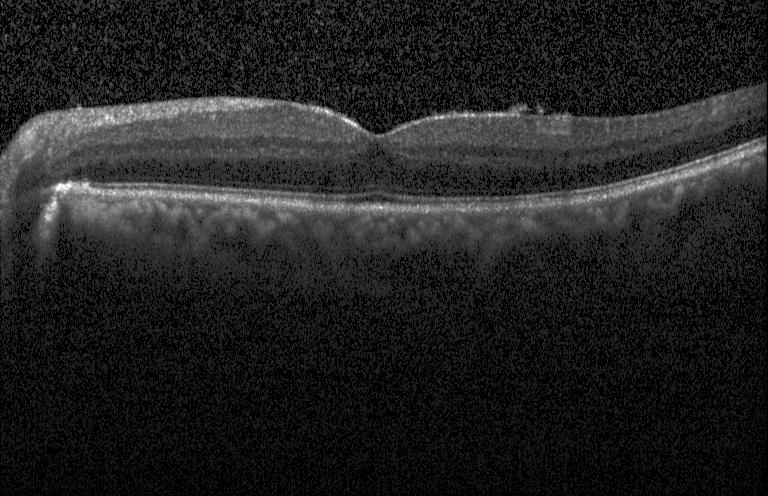

Acquired on a Heidelberg Spectralis. Retinal OCT cross-section
Finding: neither choroidal neovascularization, diabetic macular edema, nor drusen.